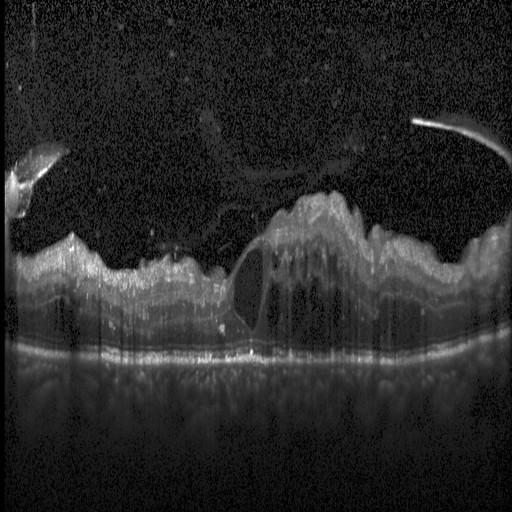
Macular OCT: DME.